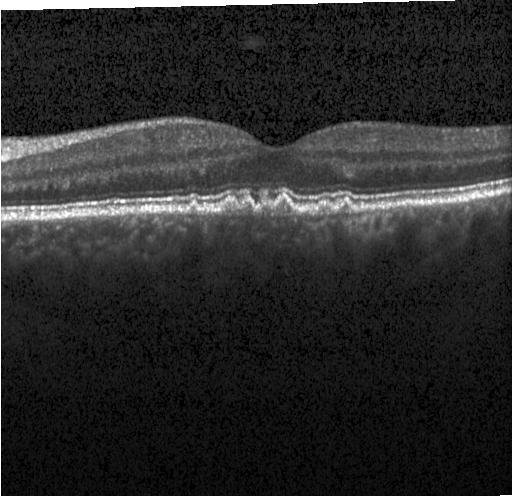 Heidelberg Spectralis. Optical coherence tomography B-scan — Impression: sub-RPE drusenoid deposits.